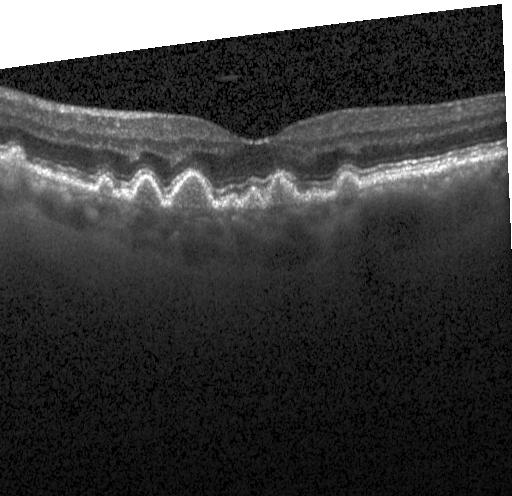 Heidelberg Spectralis OCT system · centered on the fovea · optical coherence tomography scan · spectral-domain OCT.
Drusen.